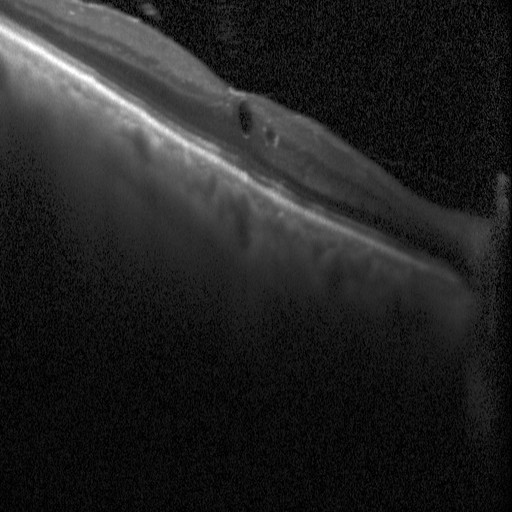

Dx: diabetic macular edema (DME).